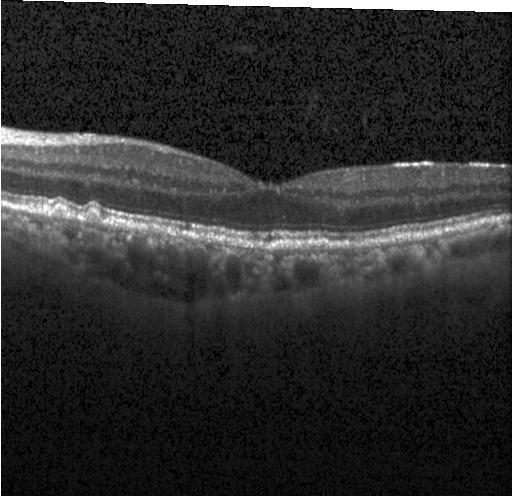 Dx: multiple drusen.